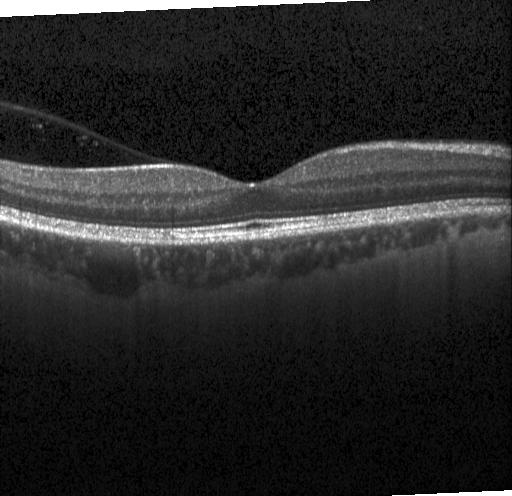
OCT scan showing no choroidal neovascularization, diabetic macular edema, or drusen.